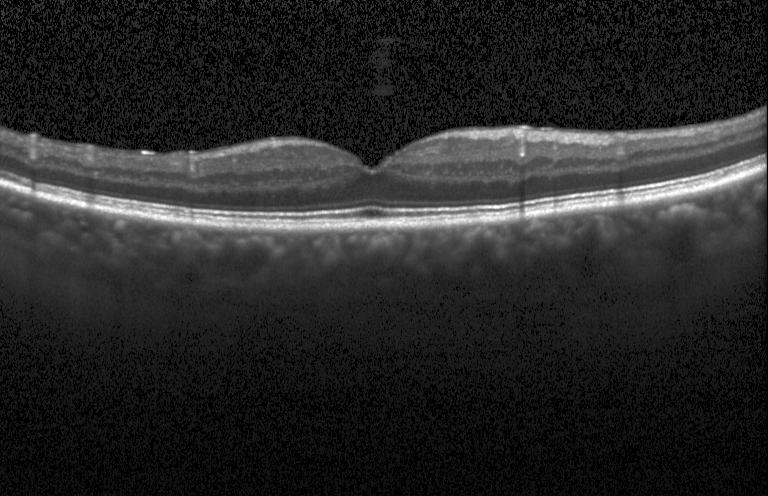

Assessment: no evidence of choroidal neovascularization, diabetic macular edema, or drusen.